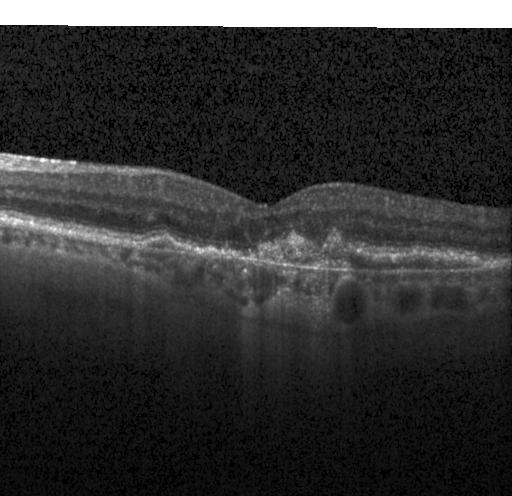
Acquired on a Heidelberg Spectralis, SD-OCT, optical coherence tomography scan, through the macula.
Finding: choroidal neovascularization.